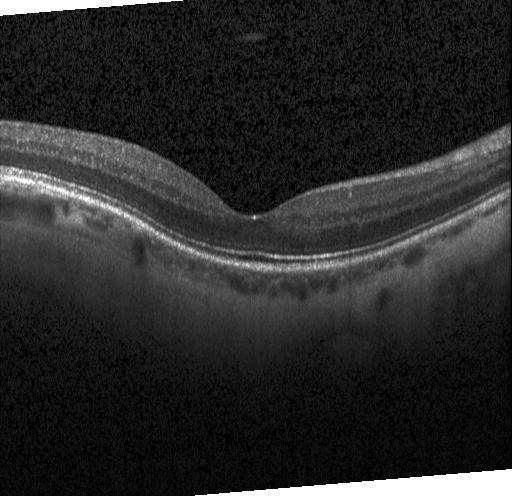

Horizontal scan through the fovea, retinal OCT B-scan — Diagnosis: neither choroidal neovascularization, diabetic macular edema, nor drusen.